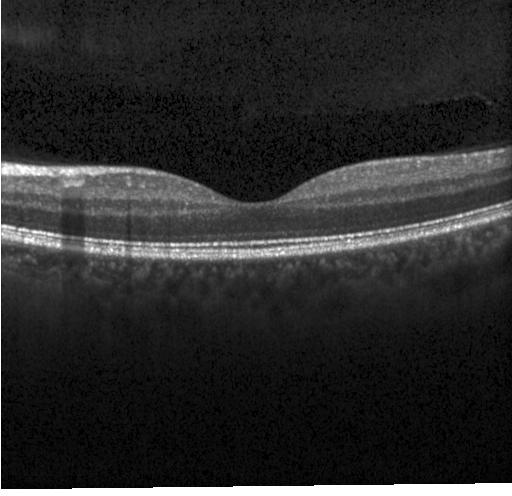
Acquired on a Heidelberg Spectralis; OCT B-scan. Diagnosis: no choroidal neovascularization, diabetic macular edema, or drusen.